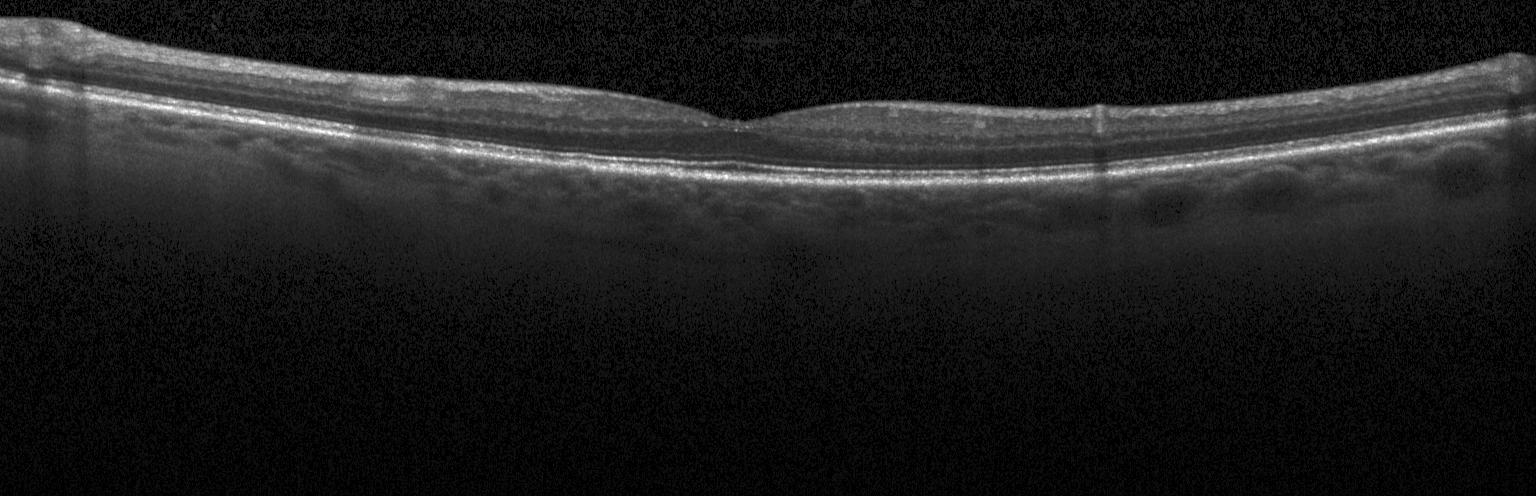

OCT line scan.
No choroidal neovascularization, diabetic macular edema, or drusen.